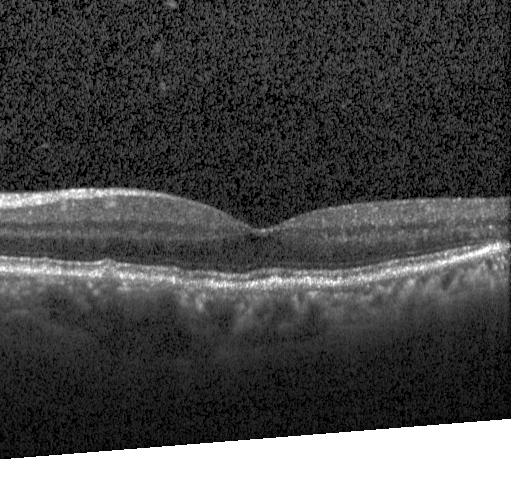
Horizontal scan through the fovea; retinal OCT cross-section.
Finding: drusen.